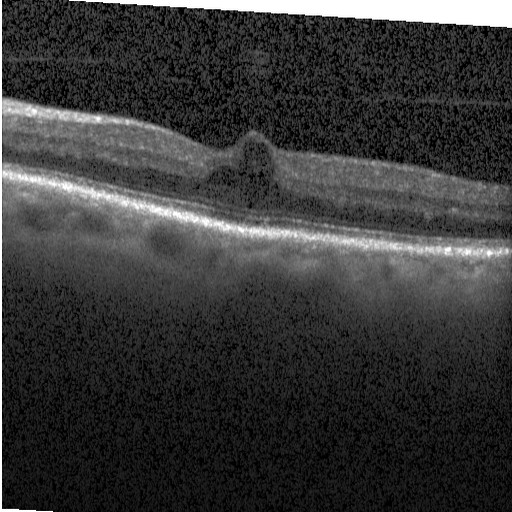
Fovea-centered · Heidelberg Spectralis OCT system · retinal OCT cross-section
This B-scan demonstrates diabetic macular edema (DME).